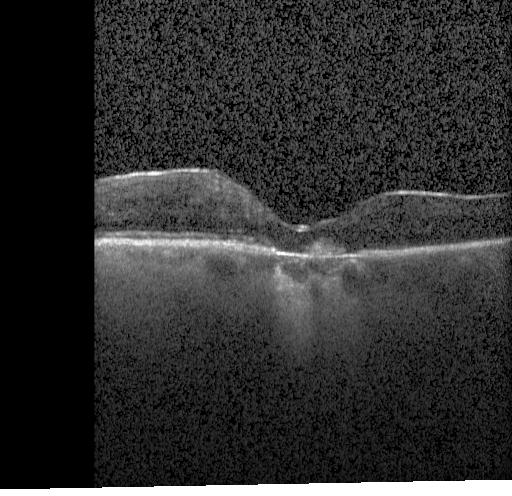 OCT B-scan, Heidelberg Spectralis OCT system.
OCT finding: a choroidal neovascular membrane.